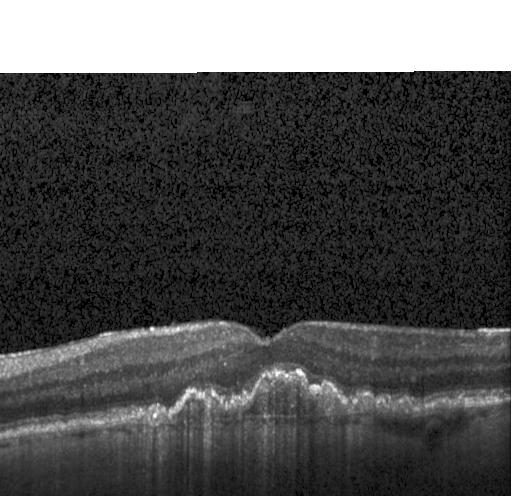
This B-scan demonstrates choroidal neovascularization (CNV).